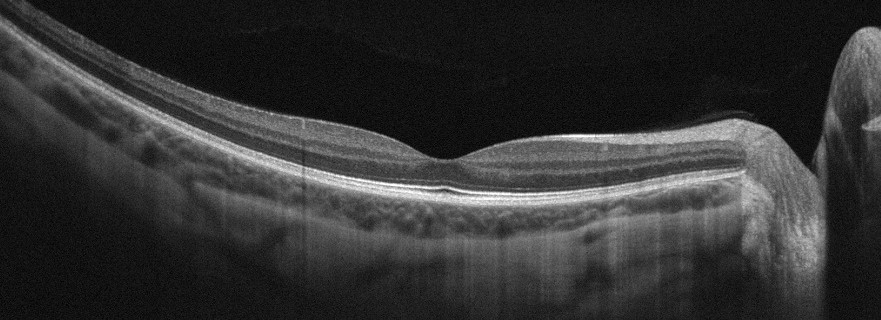

Diagnosis: absence of AMD, DME, ERM, RAO, RVO, and vitreomacular interface disease.